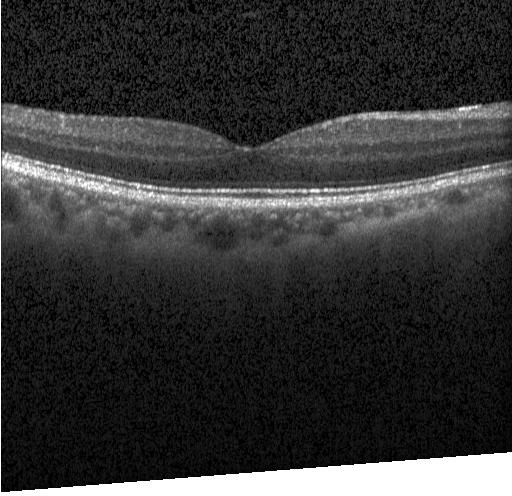

Retinal OCT cross-section — Macular OCT: no evidence of choroidal neovascularization, diabetic macular edema, or drusen.